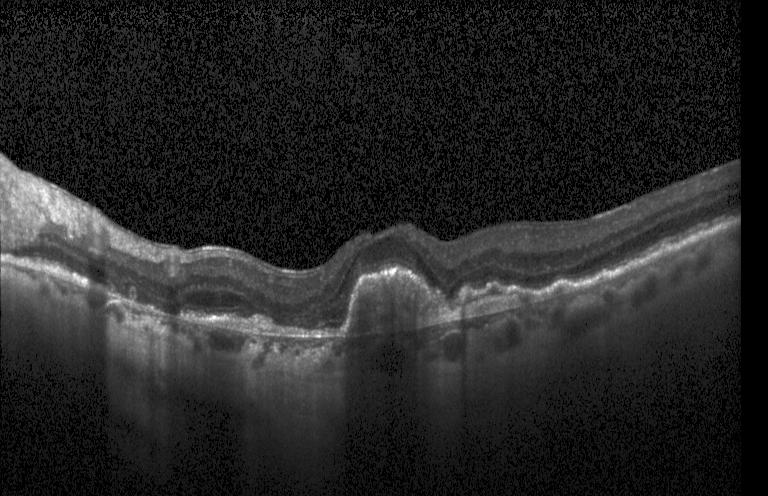
SD-OCT; horizontal scan through the fovea; retinal OCT cross-section
The scan shows a choroidal neovascular membrane.